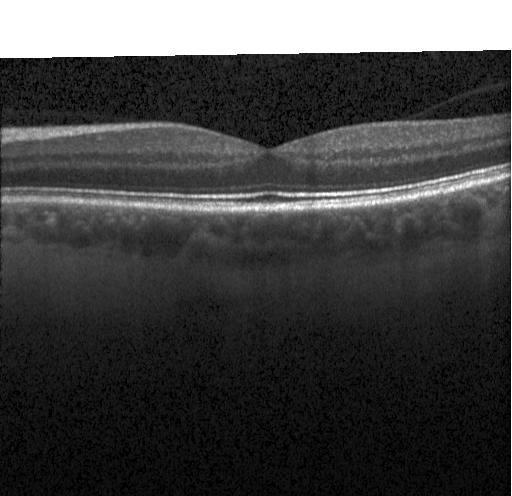 This B-scan demonstrates no CNV, no DME, and no drusen.